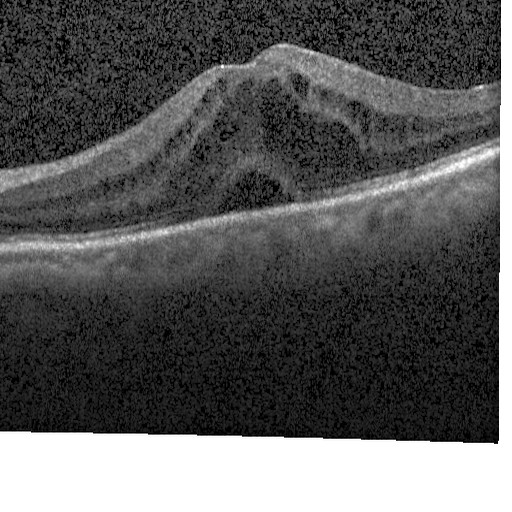
OCT line scan. Finding: diabetic macular edema (DME).